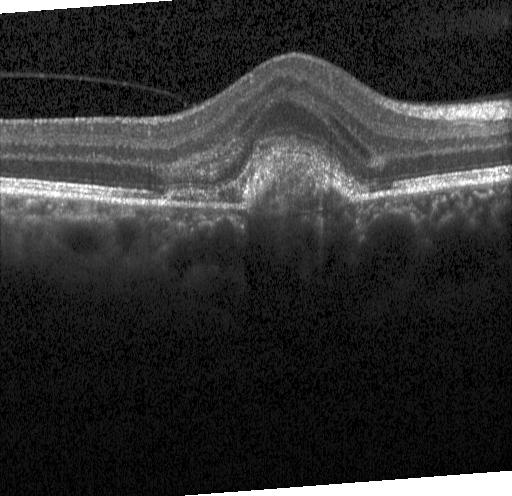
Retinal OCT cross-section showing CNV.